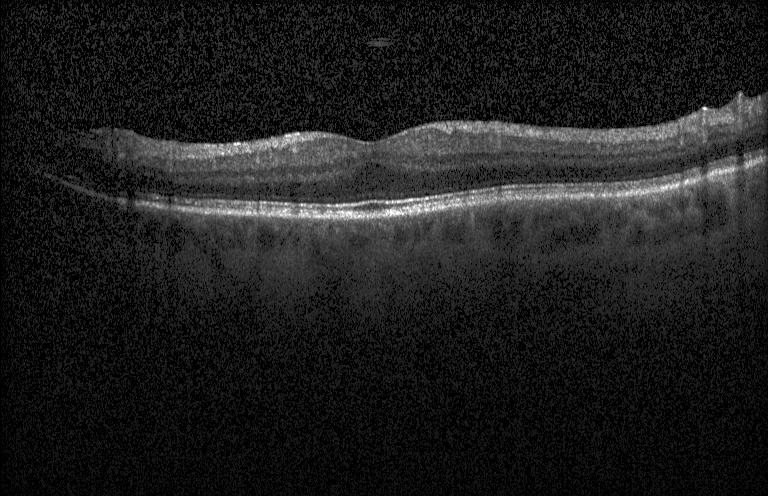
The scan shows no evidence of CNV, DME, or drusen.